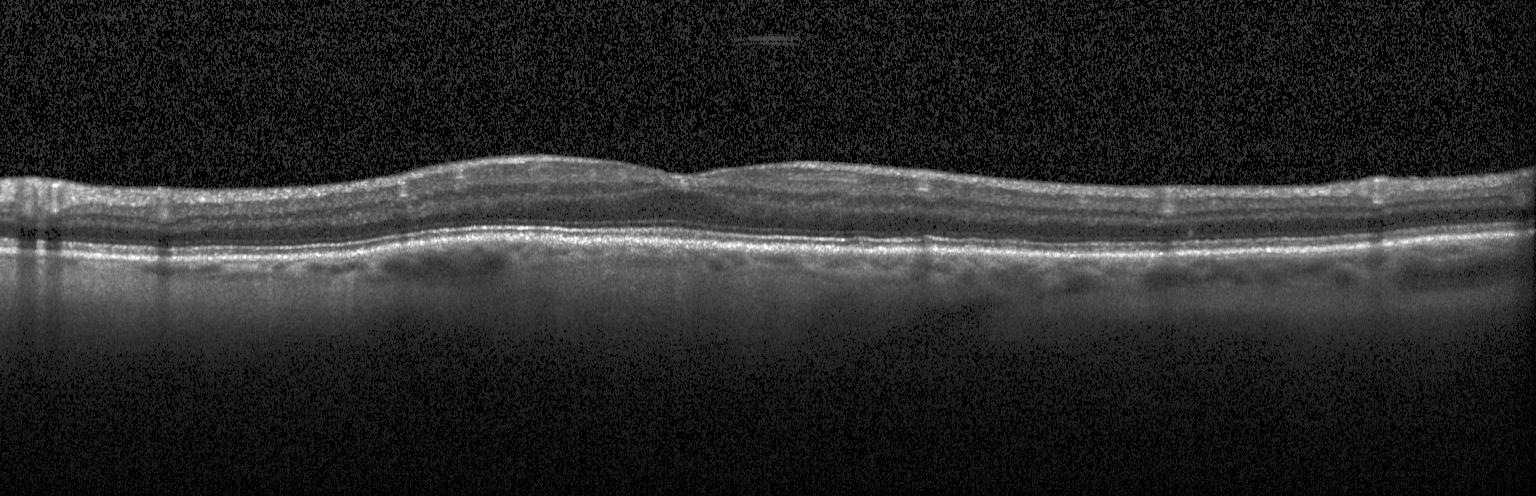
Neither CNV, DME, nor drusen.